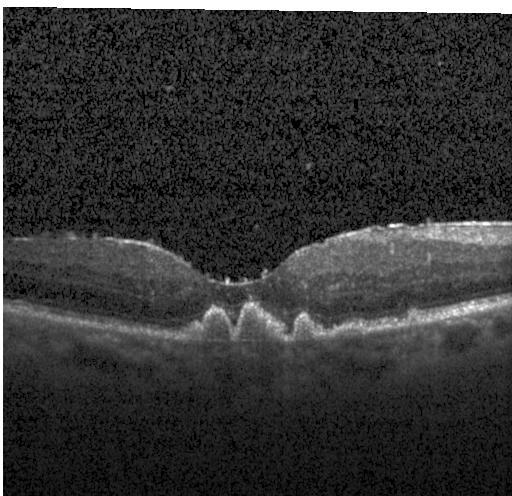

Diagnosis: sub-RPE drusenoid deposits.